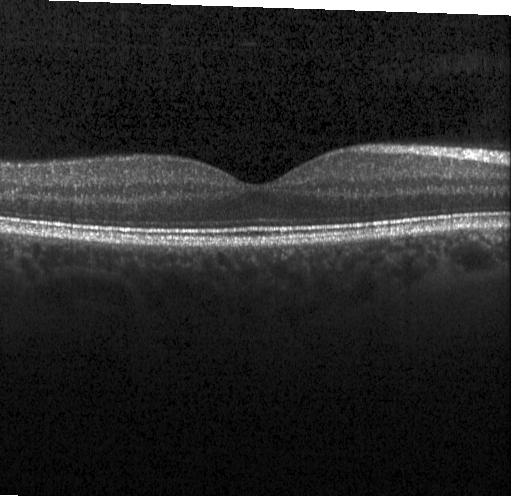
Retinal OCT B-scan, SD-OCT, Heidelberg Spectralis OCT system.
Neither choroidal neovascularization, diabetic macular edema, nor drusen.